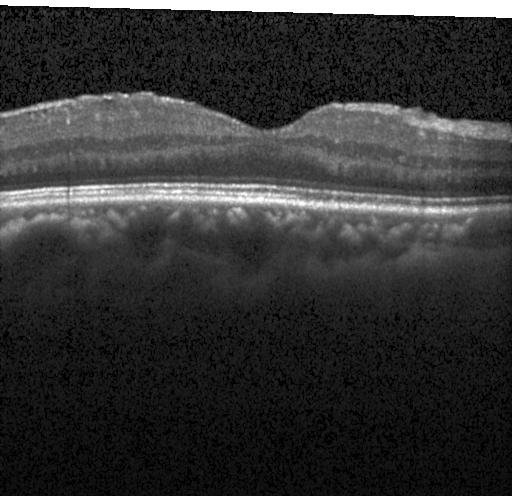
Retinal OCT cross-section · Heidelberg Spectralis · spectral-domain optical coherence tomography · through the macula. Impression: no CNV, DME, or drusen.